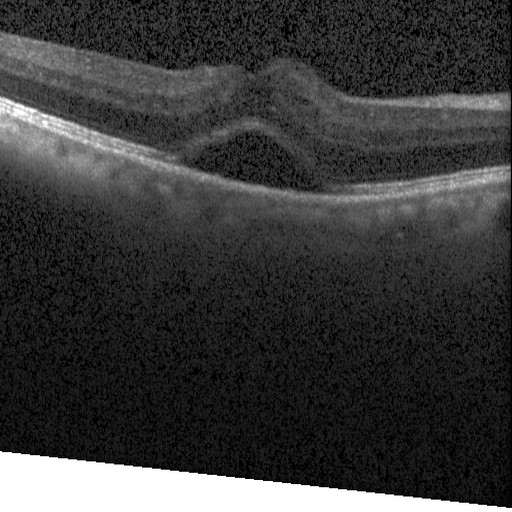
Heidelberg Spectralis; OCT line scan; spectral-domain OCT — Assessment: DME.